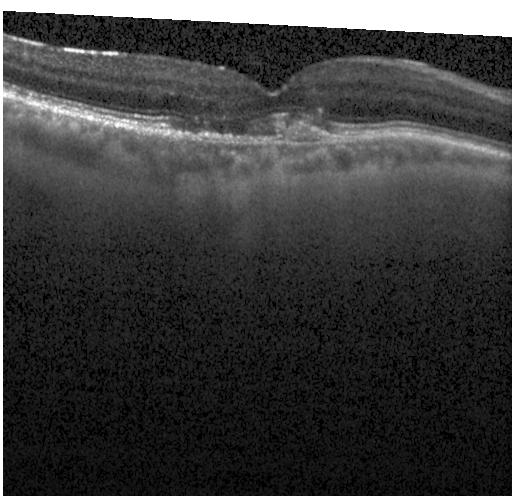

OCT B-scan.
The scan shows choroidal neovascularization (CNV).